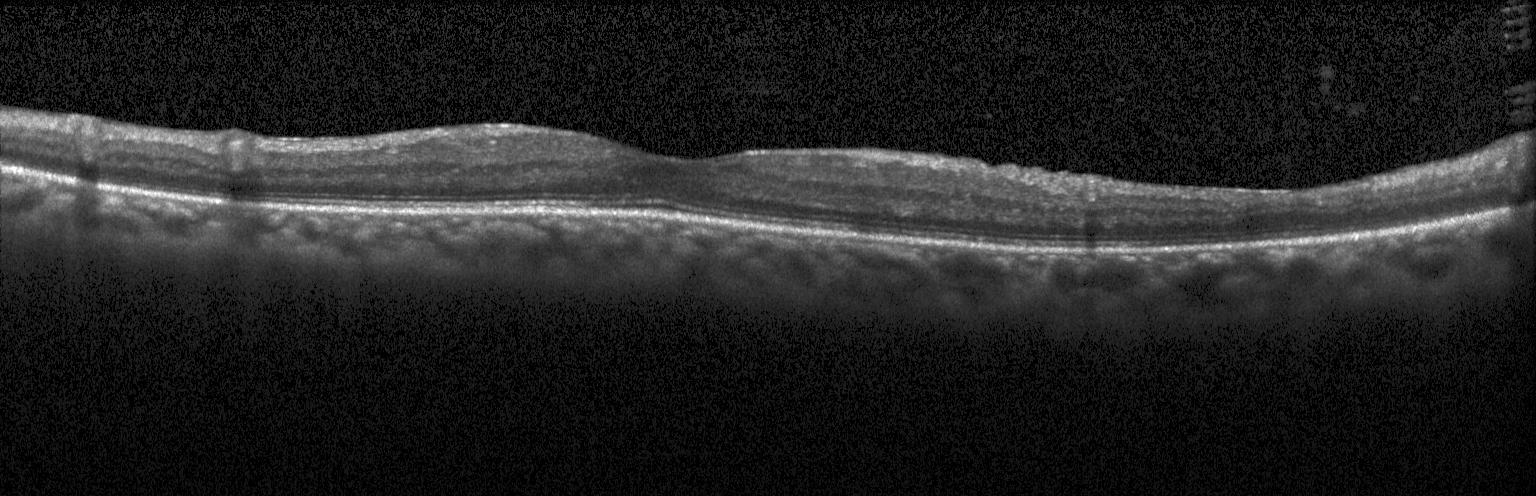

Instrument: Heidelberg Spectralis, SD-OCT, OCT B-scan.
Finding: no choroidal neovascularization, diabetic macular edema, or drusen.